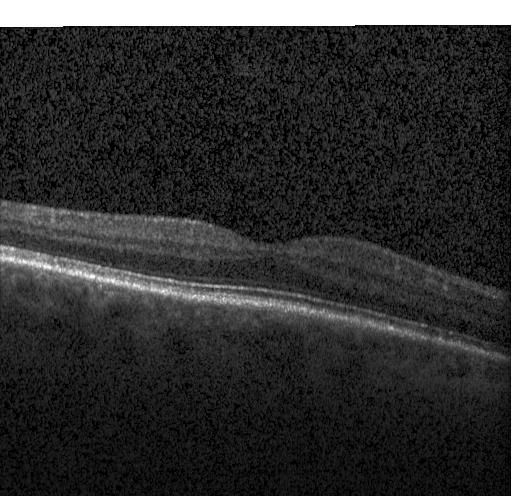 Optical coherence tomography B-scan.
Impression: no evidence of CNV, DME, or drusen.